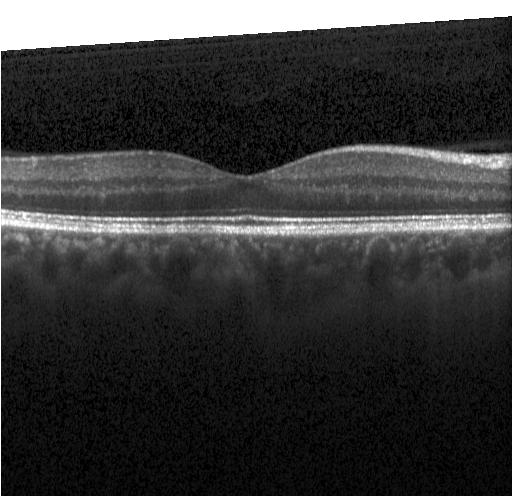
Assessment: neither choroidal neovascularization, diabetic macular edema, nor drusen.